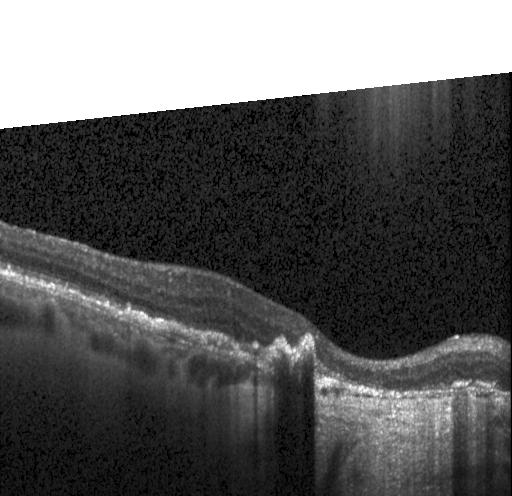

OCT B-scan — Finding: a choroidal neovascular membrane.